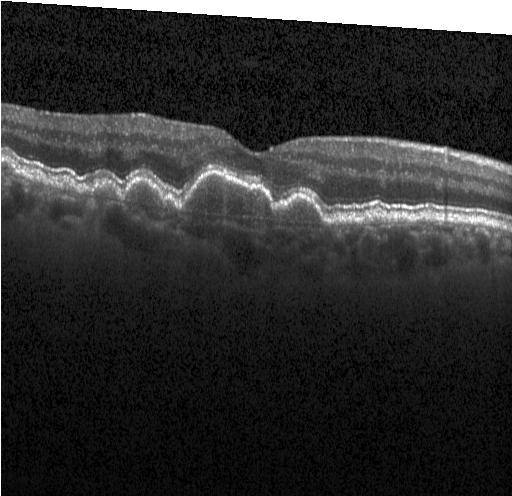

Fovea-centered, optical coherence tomography scan. Dx: drusen.